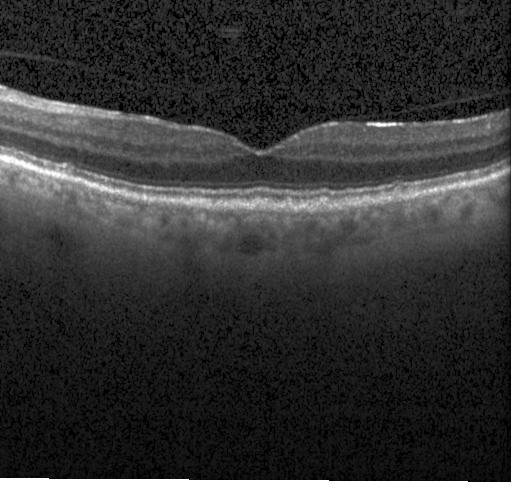
Assessment: multiple drusen.